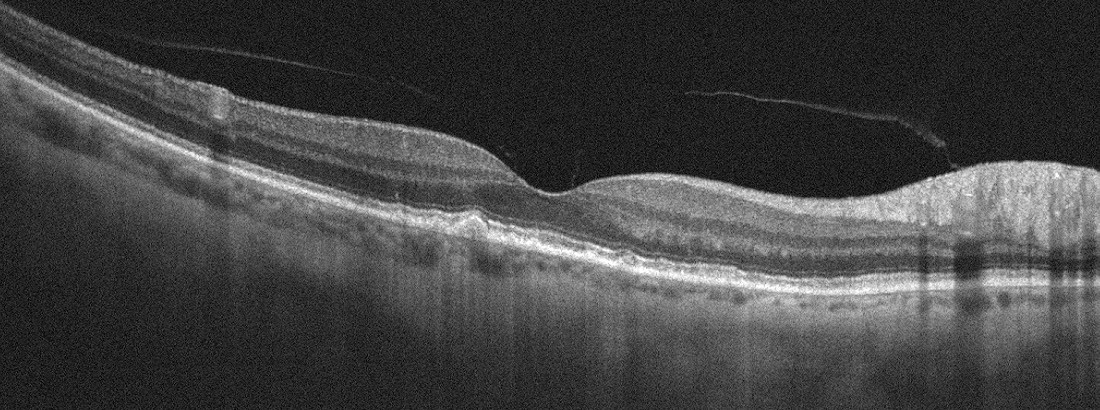

Optical coherence tomography scan; macular scan
Finding: age-related macular degeneration.